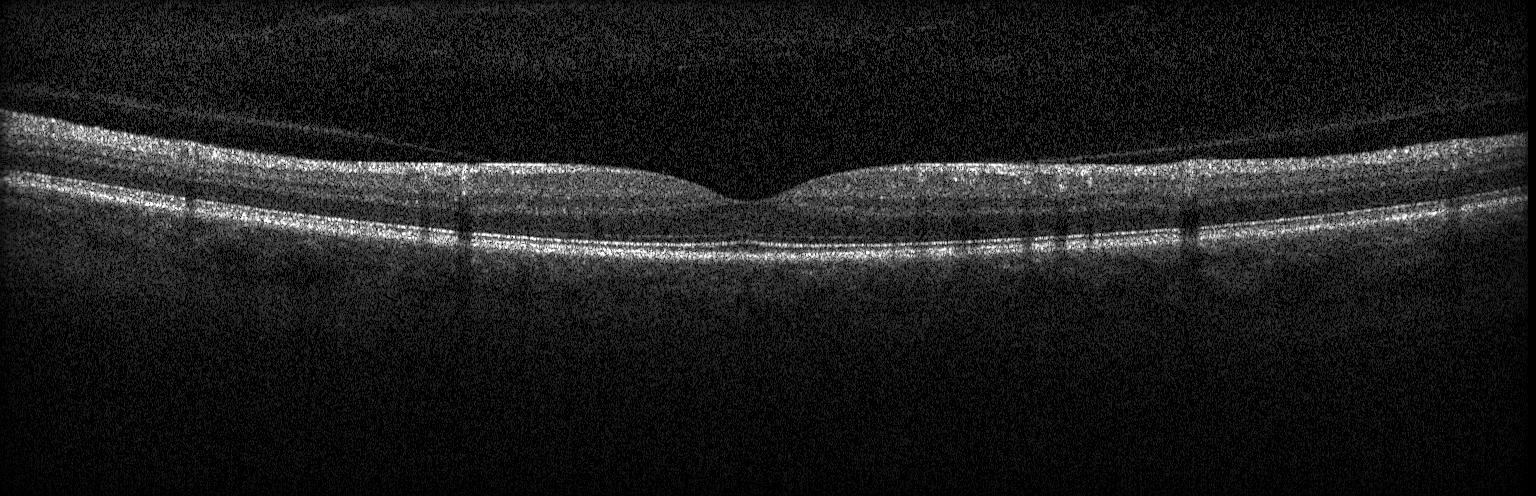

SD-OCT; optical coherence tomography scan. Impression: no choroidal neovascularization, diabetic macular edema, or drusen.